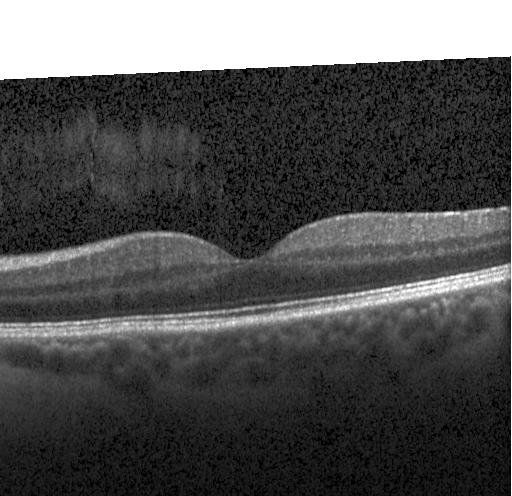
Impression: no evidence of choroidal neovascularization, diabetic macular edema, or drusen.